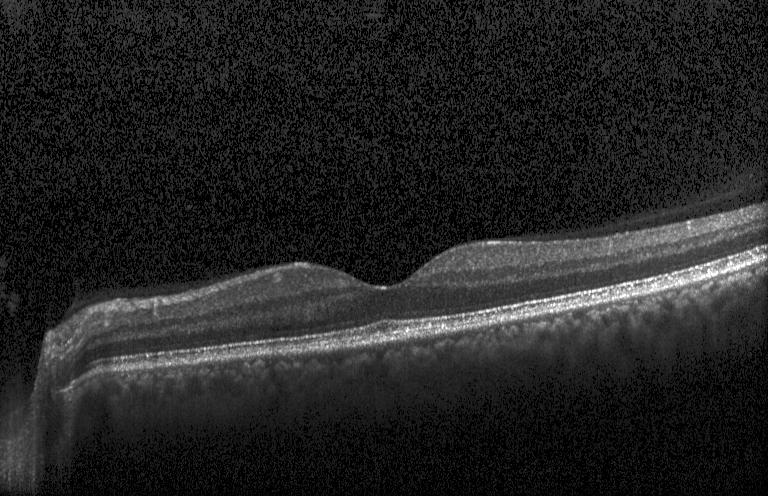

Optical coherence tomography B-scan · SD-OCT · macular scan.
Impression: no CNV, no DME, and no drusen.